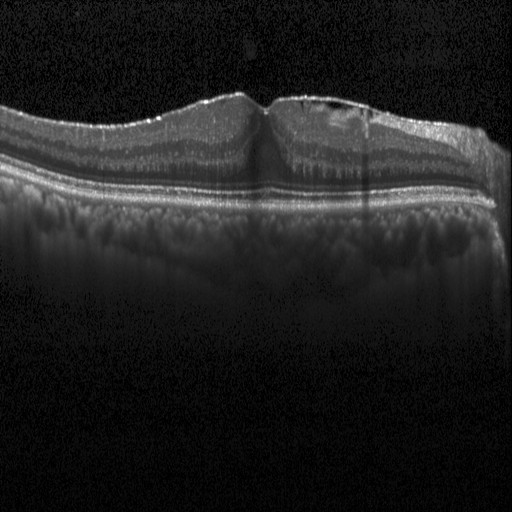 Through the macula, Heidelberg Spectralis OCT system, retinal OCT cross-section
OCT finding: diabetic macular edema (DME).